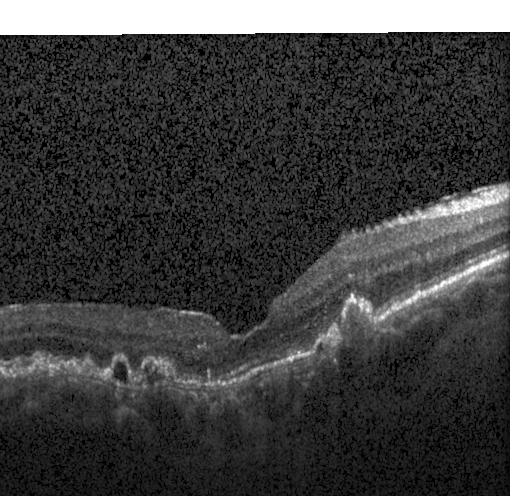

OCT scan showing a choroidal neovascular membrane.